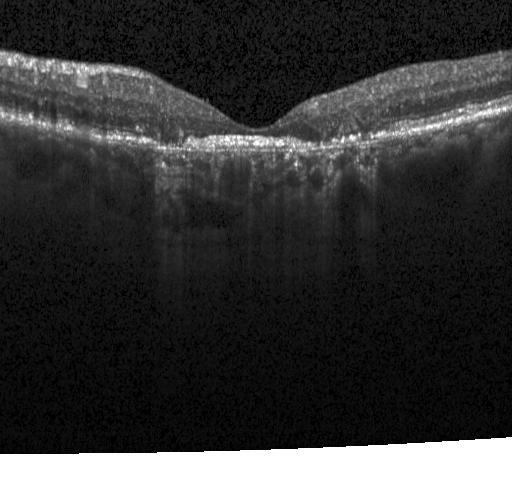 SD-OCT. OCT line scan. Macular scan.
Assessment: choroidal neovascularization.